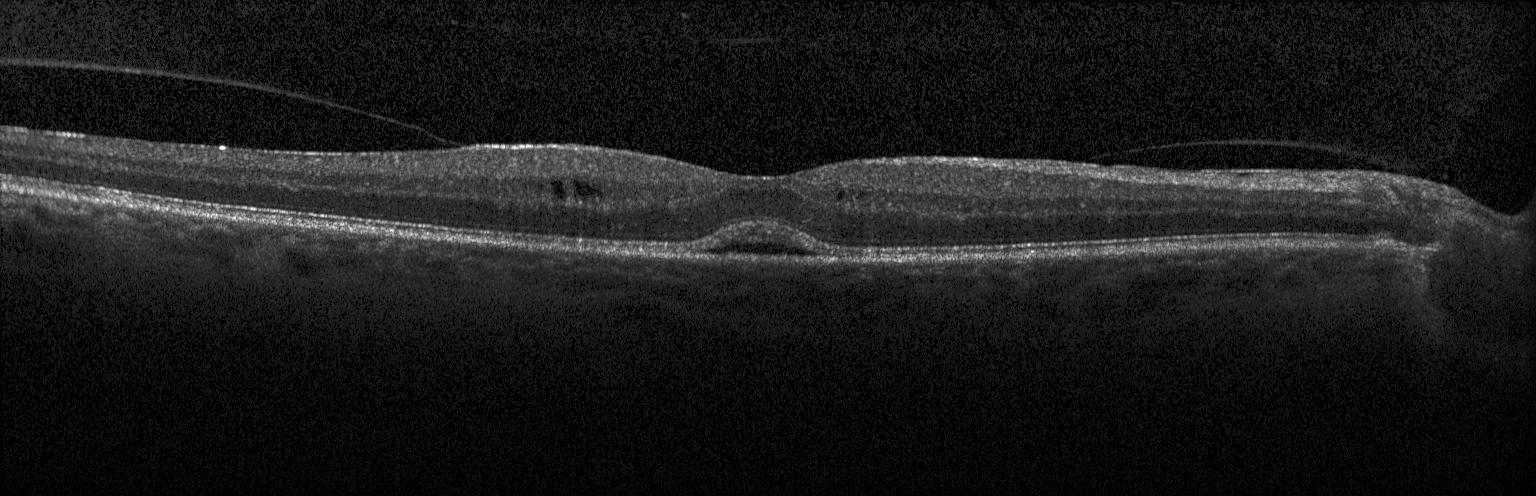

OCT B-scan.
Diabetic macular edema.